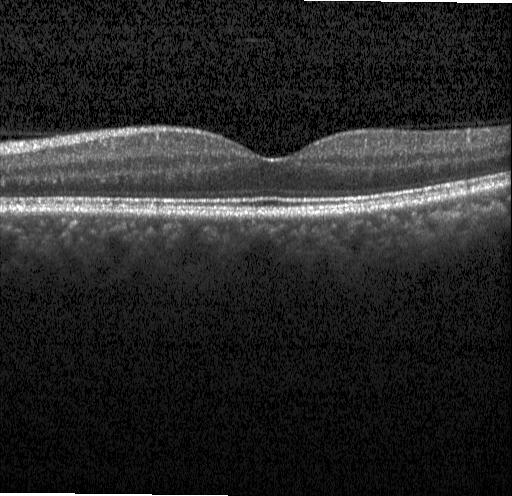 SD-OCT; acquired on a Heidelberg Spectralis; optical coherence tomography scan; macular scan. Dx: neither choroidal neovascularization, diabetic macular edema, nor drusen.